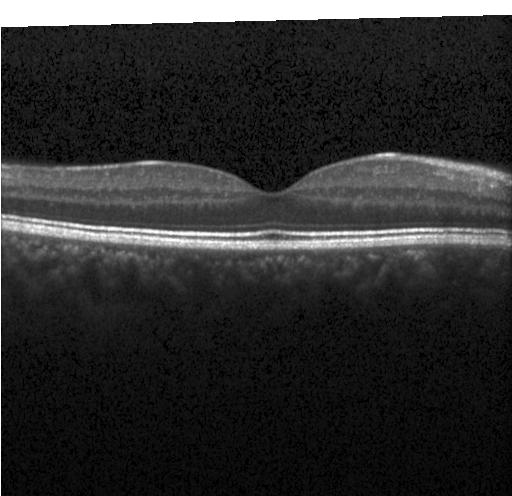

Retinal OCT cross-section. Impression: no choroidal neovascularization, no diabetic macular edema, and no drusen.